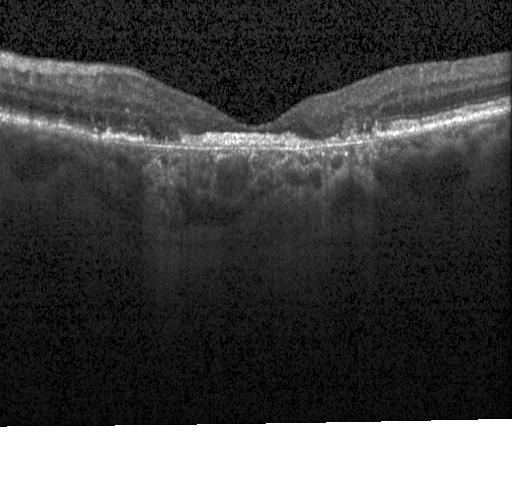 OCT line scan; Heidelberg Spectralis OCT system; SD-OCT; fovea-centered.
Finding: choroidal neovascularization (CNV).